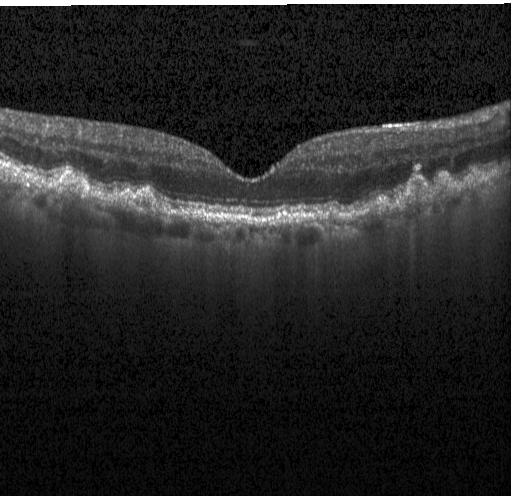 SD-OCT; centered on the fovea; optical coherence tomography scan.
Finding: sub-RPE drusenoid deposits.